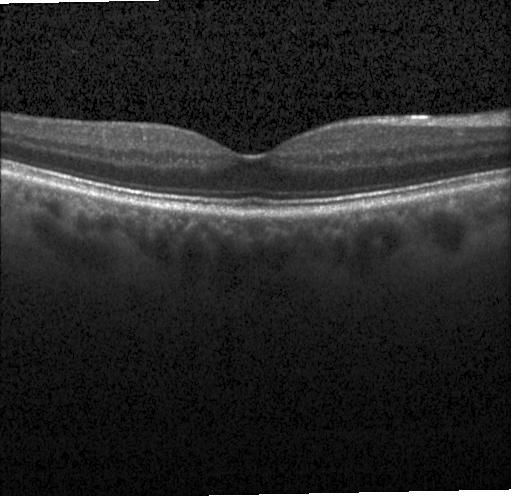

Finding: neither choroidal neovascularization, diabetic macular edema, nor drusen.